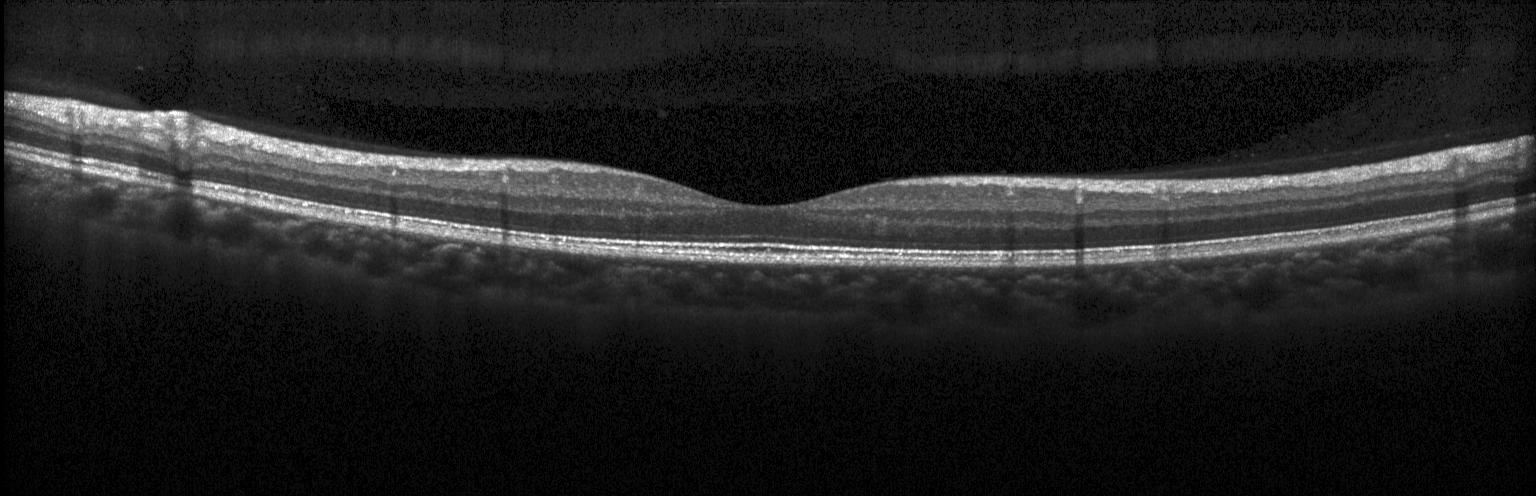
Acquired on a Heidelberg Spectralis; OCT line scan; centered on the fovea; SD-OCT
No CNV, no DME, and no drusen.